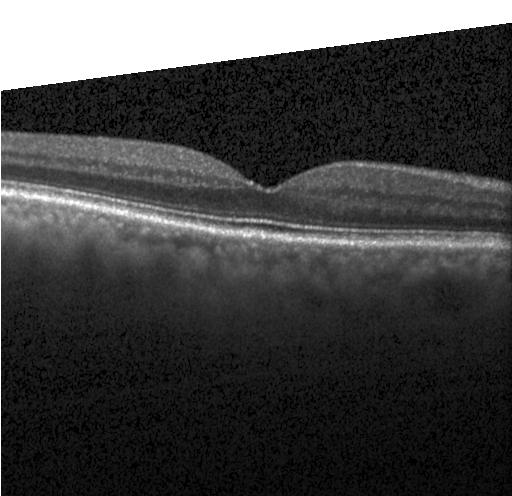

Spectral-domain OCT B-scan: no choroidal neovascularization, diabetic macular edema, or drusen.